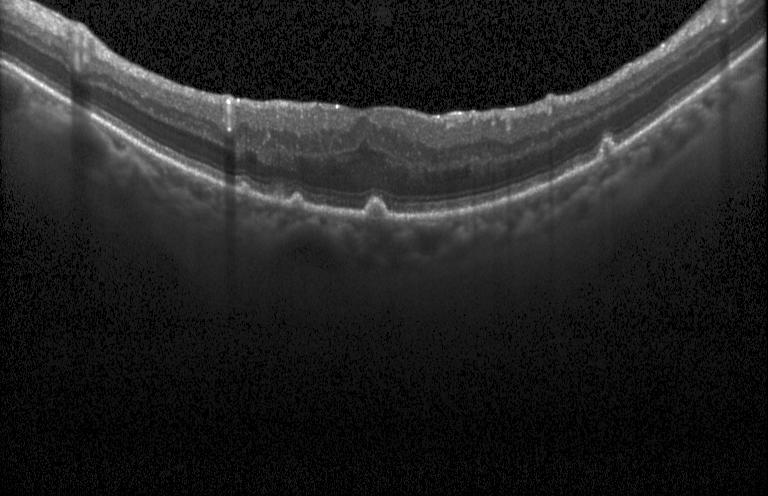 Macular scan, spectral-domain OCT, Heidelberg Spectralis, OCT line scan — Impression: multiple drusen.